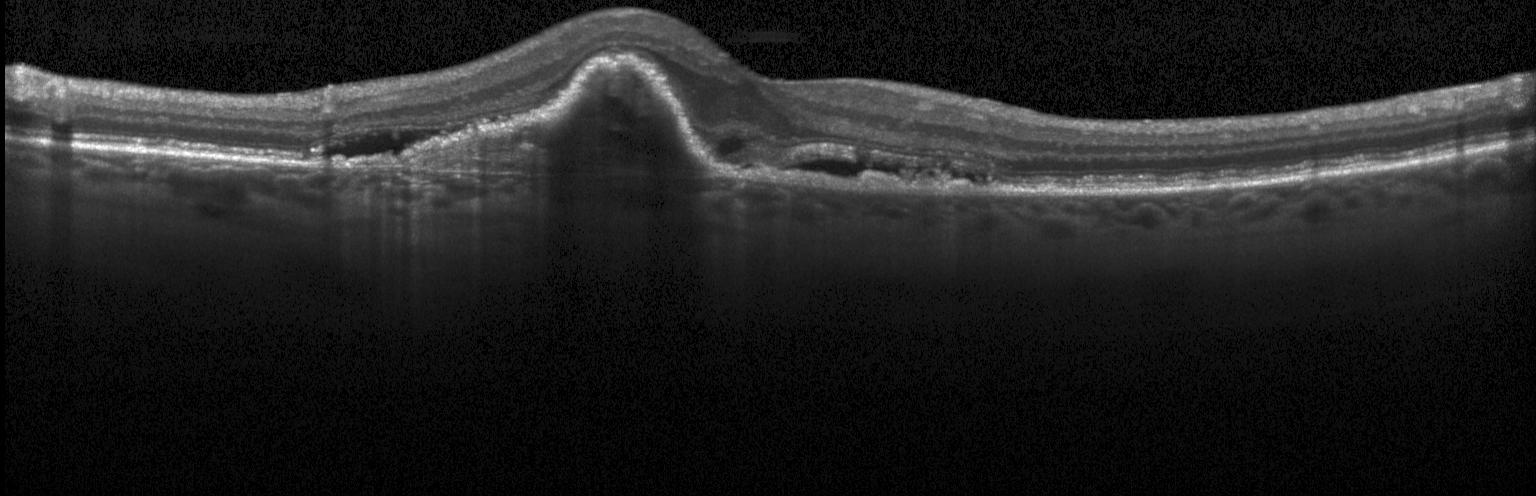
Through the macula. OCT line scan.
Macular OCT: CNV.